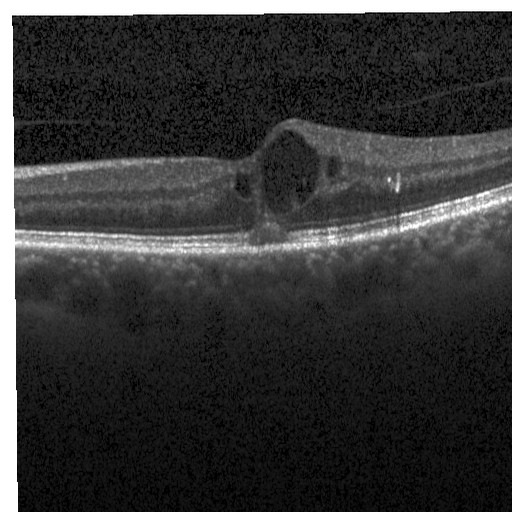

Macular scan; retinal OCT B-scan; acquired on a Heidelberg Spectralis — Diabetic macular edema (DME).